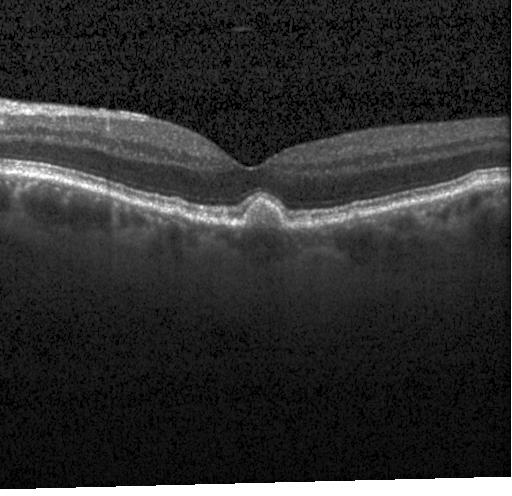
Macular OCT: sub-RPE drusenoid deposits.